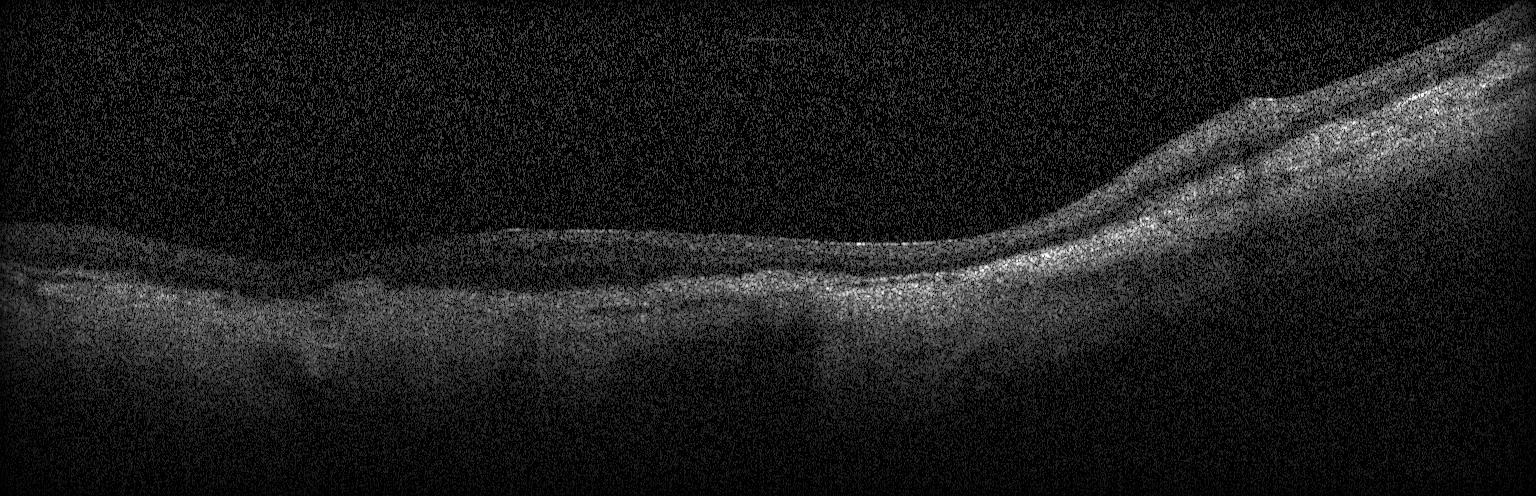
OCT line scan; centered on the fovea.
Finding: CNV.